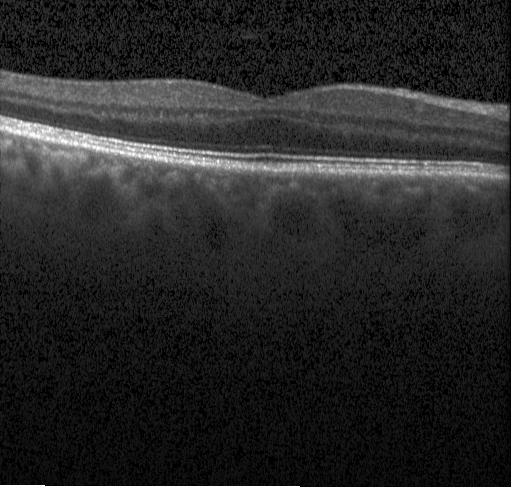 Retinal OCT B-scan. Acquired on a Heidelberg Spectralis
Assessment: no choroidal neovascularization, diabetic macular edema, or drusen.